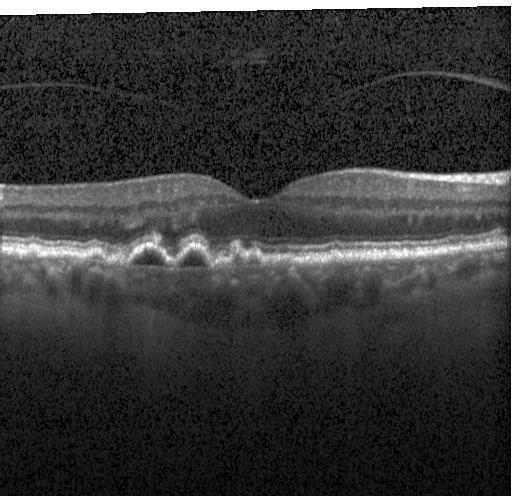 Retinal OCT cross-section. Centered on the fovea. Acquired on a Heidelberg Spectralis.
Impression: choroidal neovascularization.